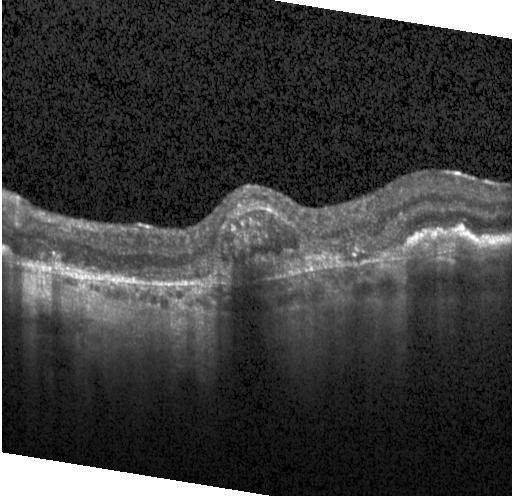
Finding: choroidal neovascularization.